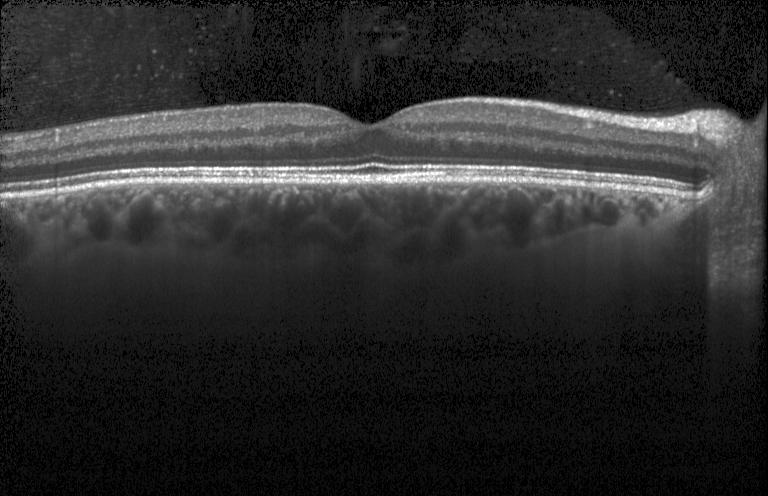
OCT scan showing no choroidal neovascularization, no diabetic macular edema, and no drusen.